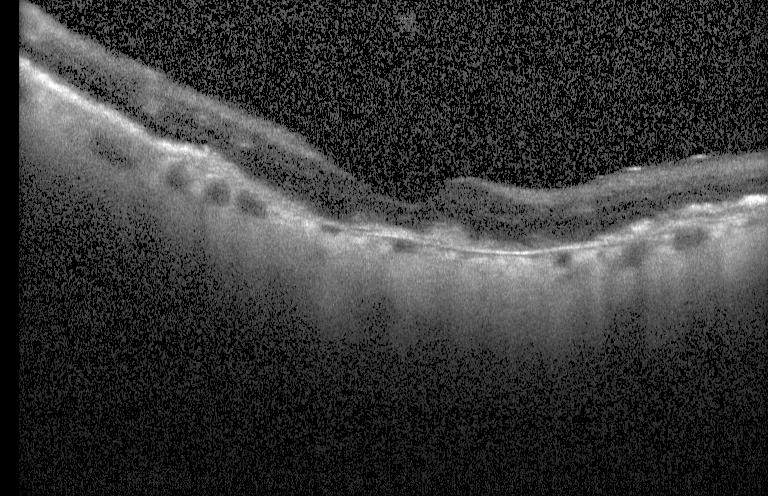 Fovea-centered; OCT B-scan
This B-scan demonstrates a choroidal neovascular membrane.